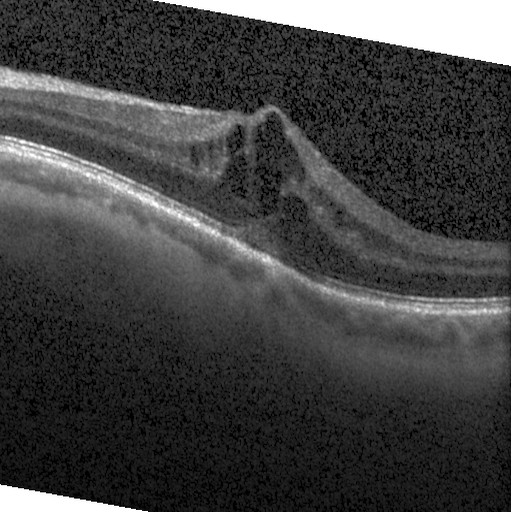
Diagnosis: DME.